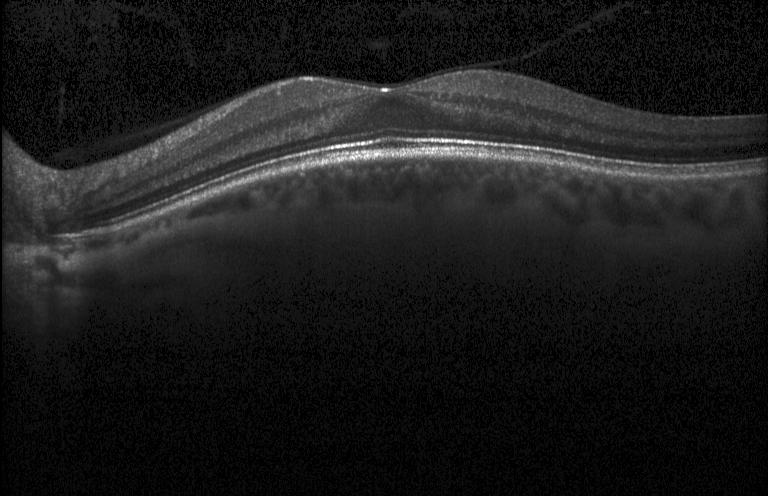
This B-scan demonstrates no choroidal neovascularization, no diabetic macular edema, and no drusen.